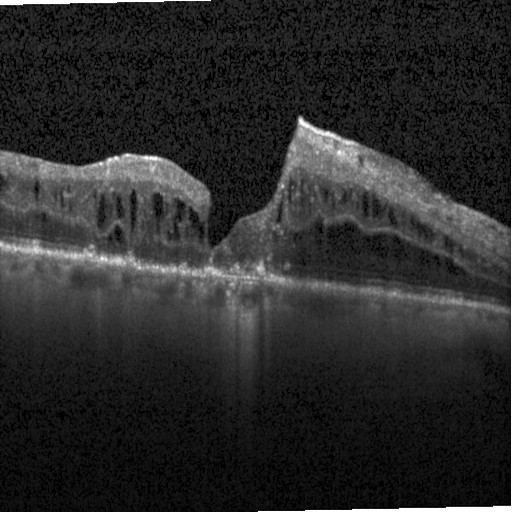
OCT B-scan showing diabetic macular edema (DME).